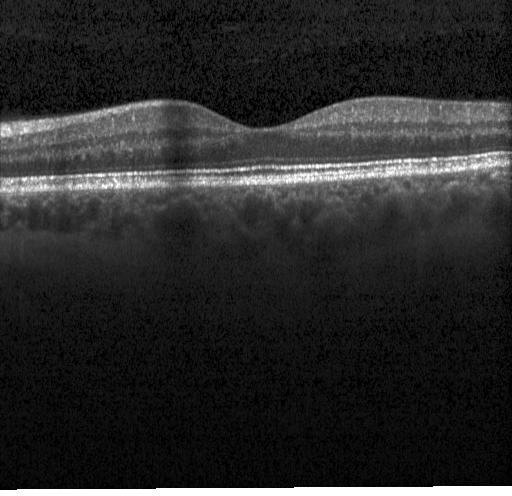
Macular scan; spectral-domain OCT; instrument: Heidelberg Spectralis; retinal OCT cross-section — Finding: no evidence of CNV, DME, or drusen.